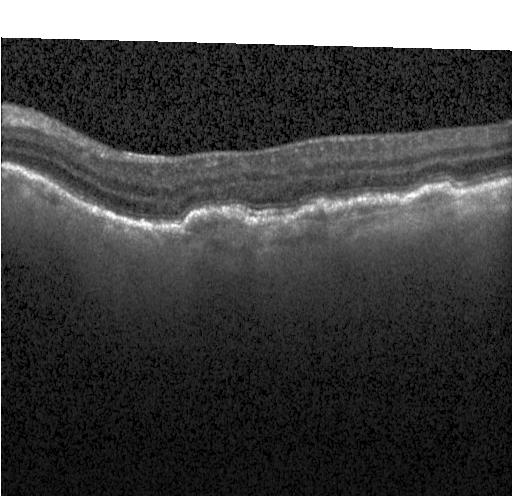
Retinal OCT B-scan; centered on the fovea. Impression: choroidal neovascularization (CNV).